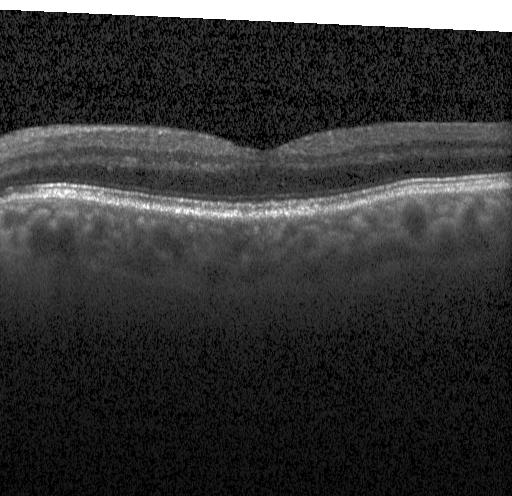 Retinal OCT cross-section. Heidelberg Spectralis. Spectral-domain OCT. Macular scan.
Impression: neither CNV, DME, nor drusen.